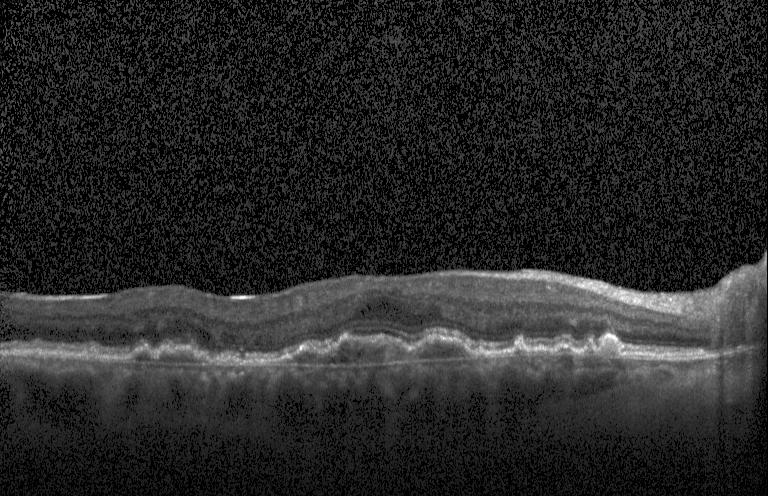 Macular OCT: a choroidal neovascular membrane.